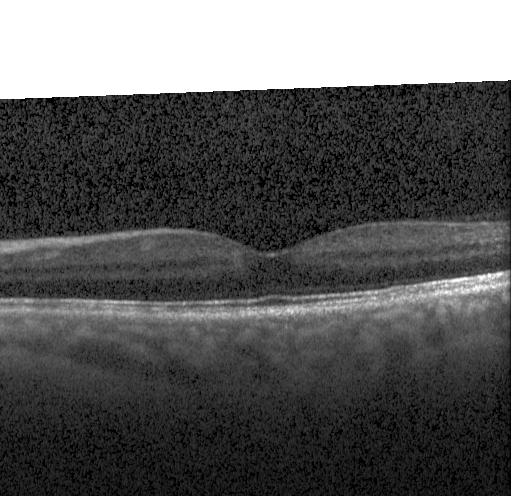

OCT finding: no CNV, no DME, and no drusen.